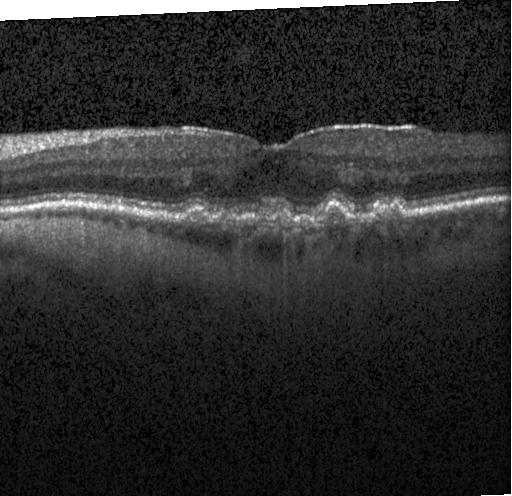
OCT finding: sub-RPE drusenoid deposits.